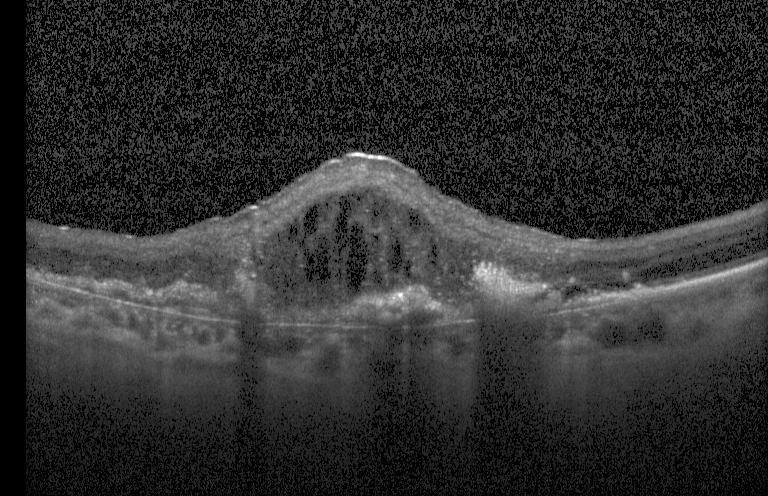

Diagnosis: a choroidal neovascular membrane.